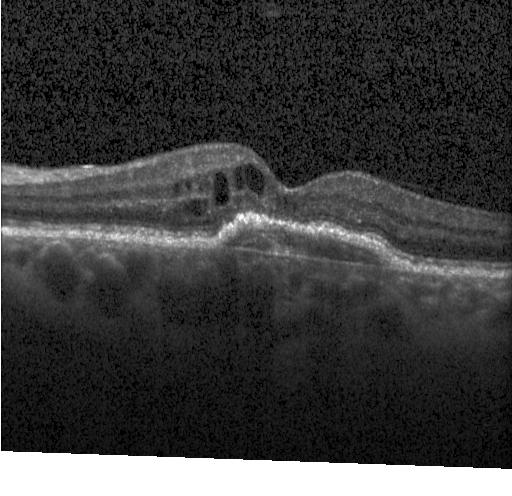 OCT B-scan — Impression: a choroidal neovascular membrane.